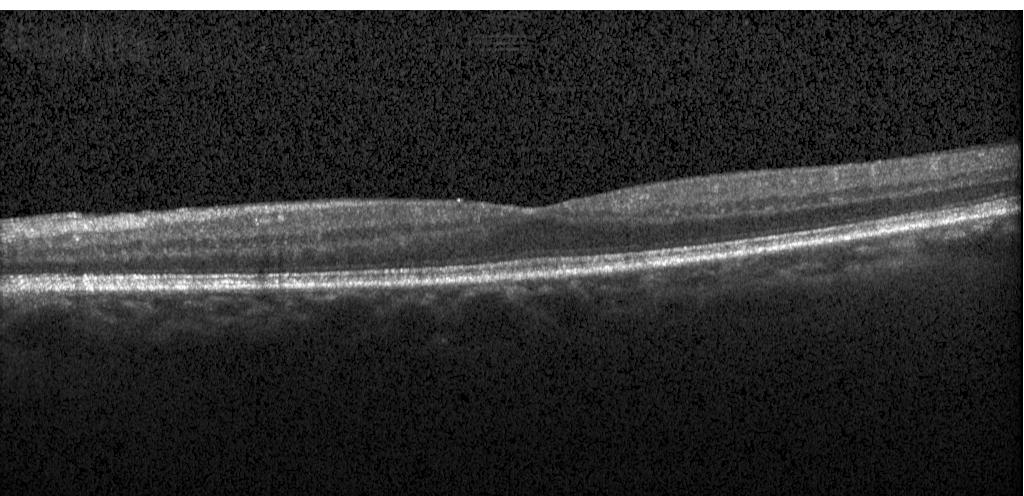 OCT B-scan; macular scan; instrument: Heidelberg Spectralis; spectral-domain OCT — Finding: no choroidal neovascularization, diabetic macular edema, or drusen.